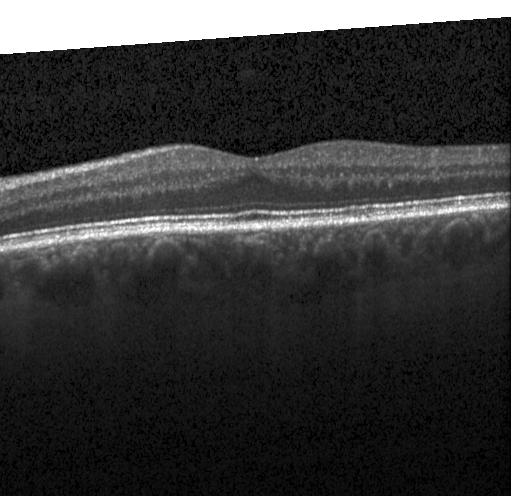 Instrument: Heidelberg Spectralis. OCT line scan — Finding: no evidence of CNV, DME, or drusen.